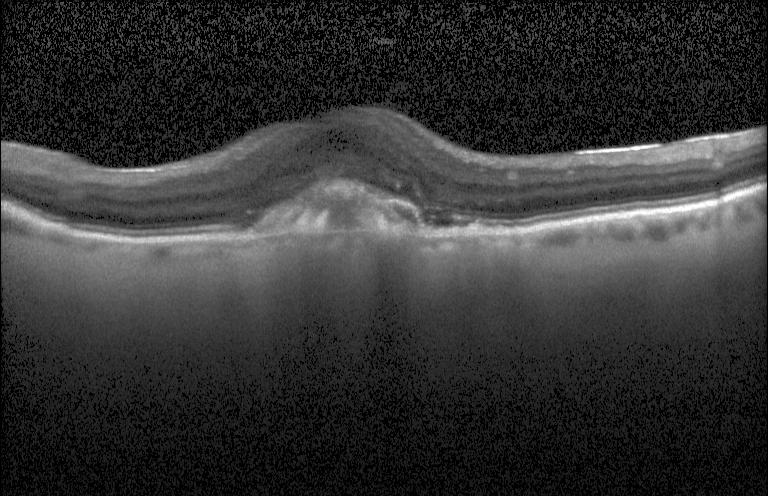 Retinal OCT B-scan · horizontal scan through the fovea. The scan shows CNV.